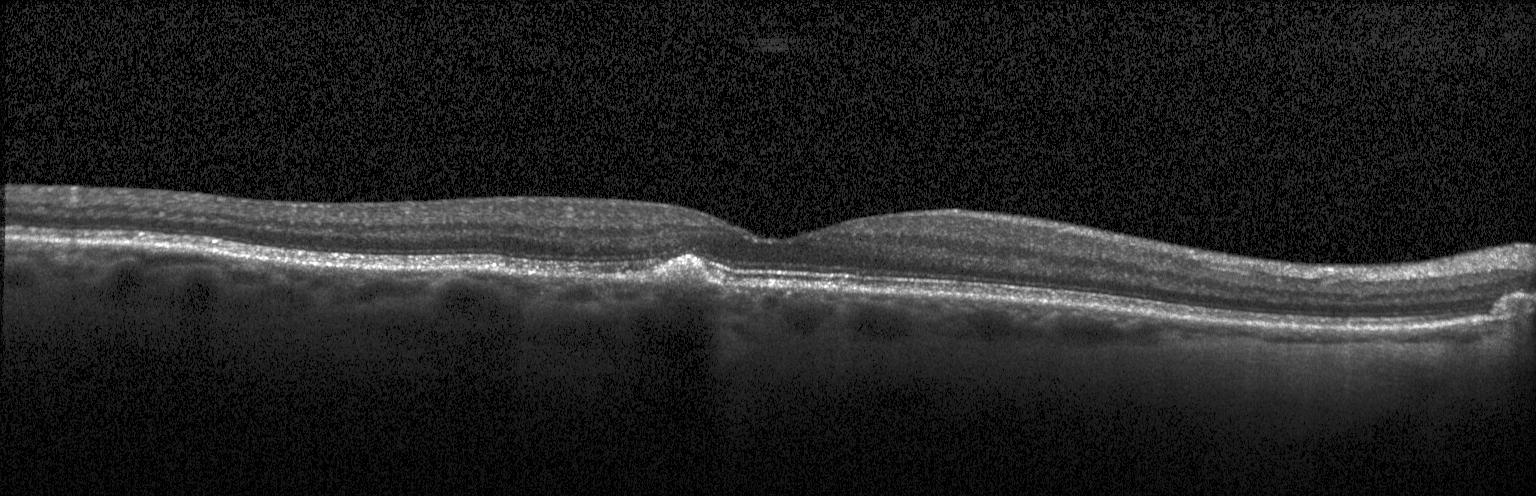

Macular scan; spectral-domain optical coherence tomography; retinal OCT cross-section; acquired on a Heidelberg Spectralis — Assessment: drusen.